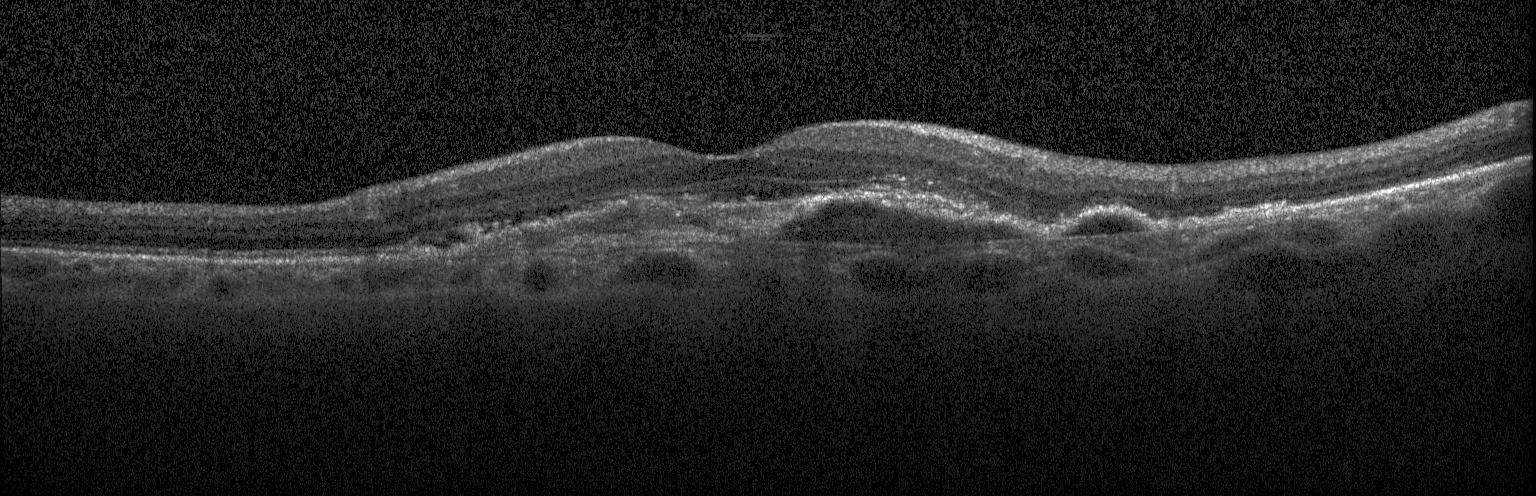
Diagnosis: CNV.